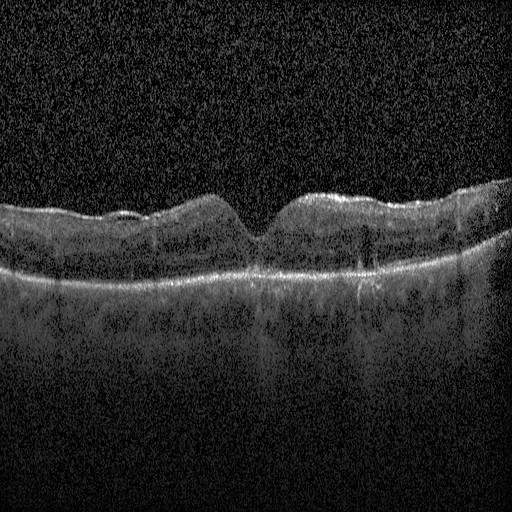 Optical coherence tomography scan. Finding: DME.